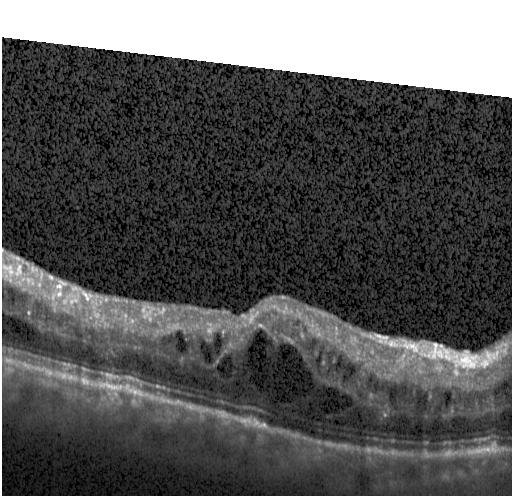

Finding: diabetic macular edema.